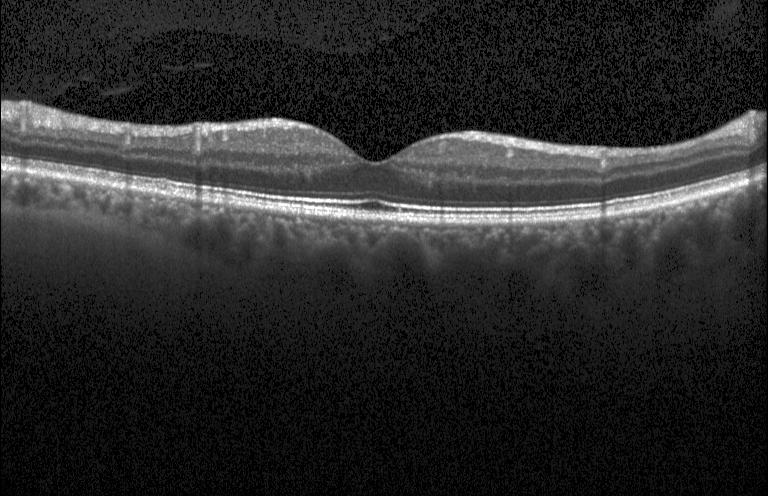
Optical coherence tomography scan
OCT finding: no CNV, no DME, and no drusen.